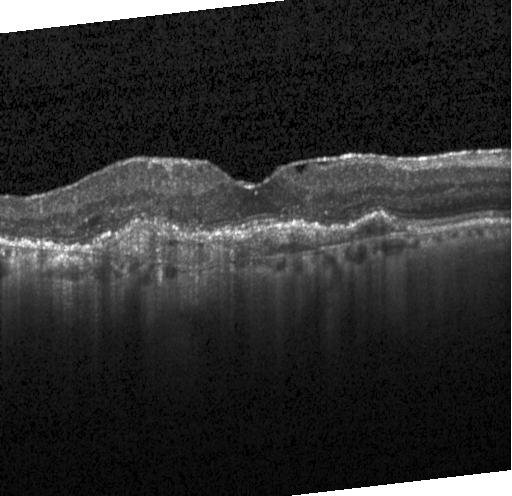

Macular scan; Heidelberg Spectralis OCT system; retinal OCT B-scan; SD-OCT. Assessment: choroidal neovascularization.